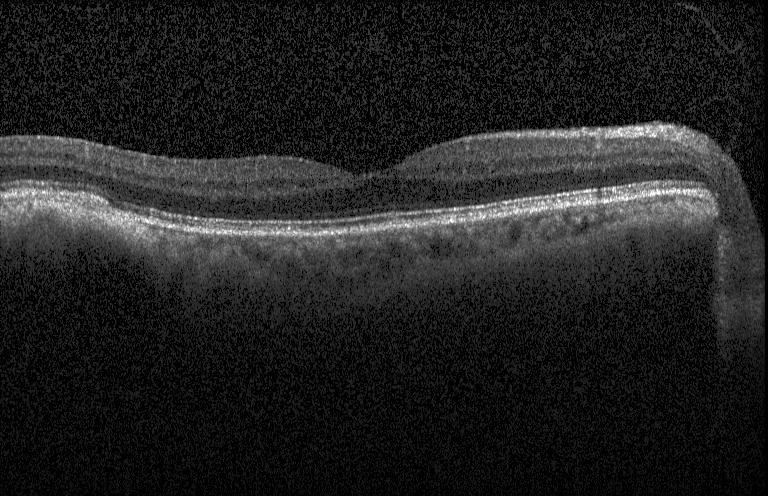
Heidelberg Spectralis OCT system, spectral-domain optical coherence tomography, retinal OCT cross-section.
This B-scan demonstrates no evidence of choroidal neovascularization, diabetic macular edema, or drusen.